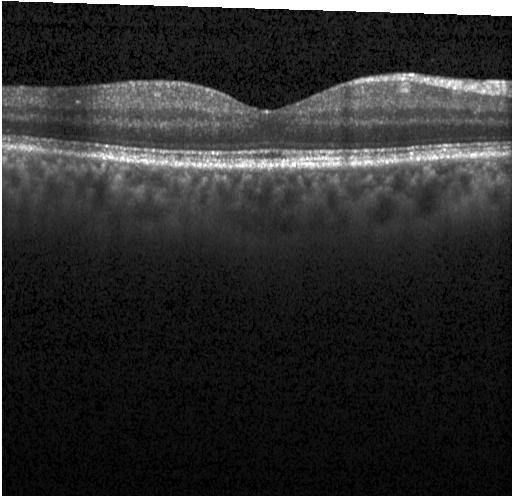
Heidelberg Spectralis. Macular scan. SD-OCT. OCT line scan.
Finding: no evidence of choroidal neovascularization, diabetic macular edema, or drusen.